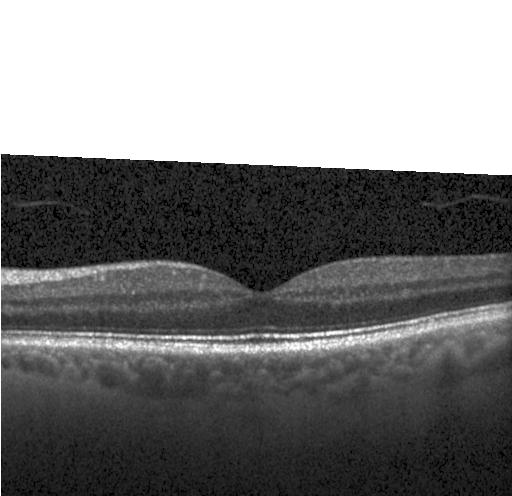
Through the macula. Spectral-domain optical coherence tomography. OCT B-scan. Macular OCT: no choroidal neovascularization, diabetic macular edema, or drusen.